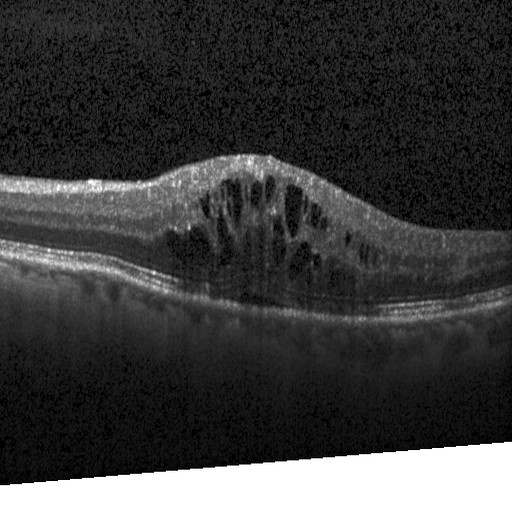
Macular scan, optical coherence tomography B-scan, Heidelberg Spectralis — Macular OCT: diabetic macular edema.